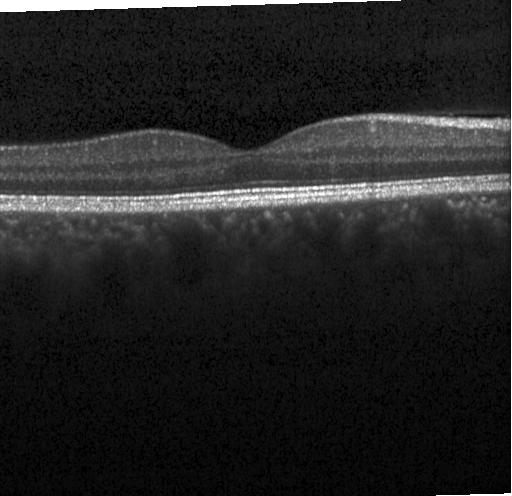
OCT B-scan.
Dx: neither choroidal neovascularization, diabetic macular edema, nor drusen.